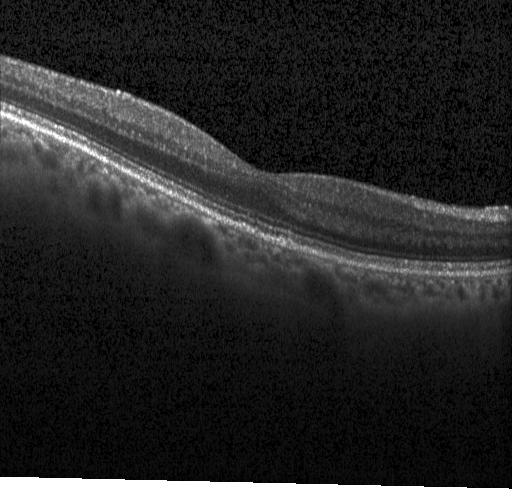

Macular scan, optical coherence tomography scan.
This B-scan demonstrates no choroidal neovascularization, no diabetic macular edema, and no drusen.